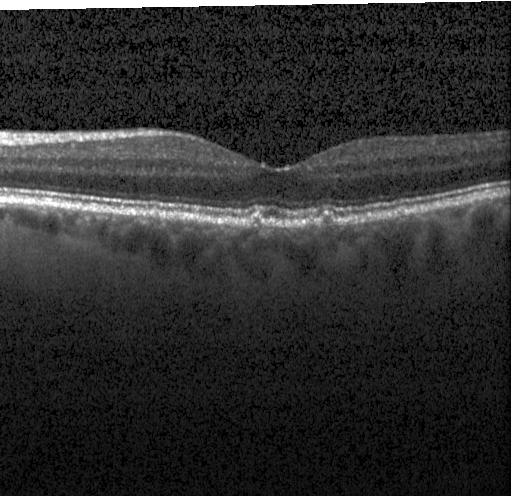 Finding: multiple drusen.